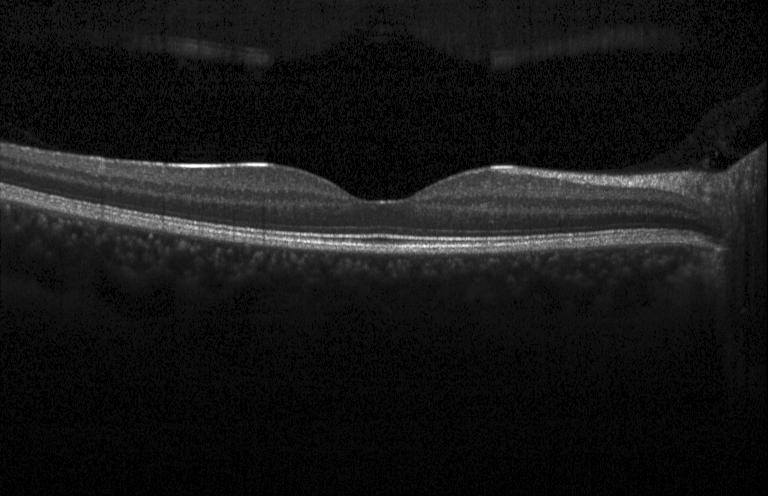
OCT line scan; Heidelberg Spectralis OCT system
Assessment: no evidence of CNV, DME, or drusen.